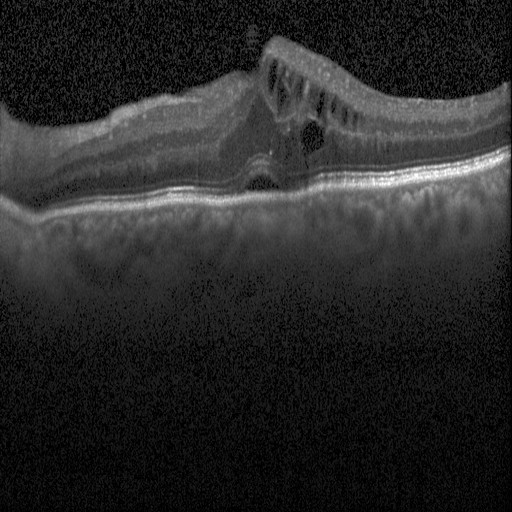 Finding: diabetic macular edema.